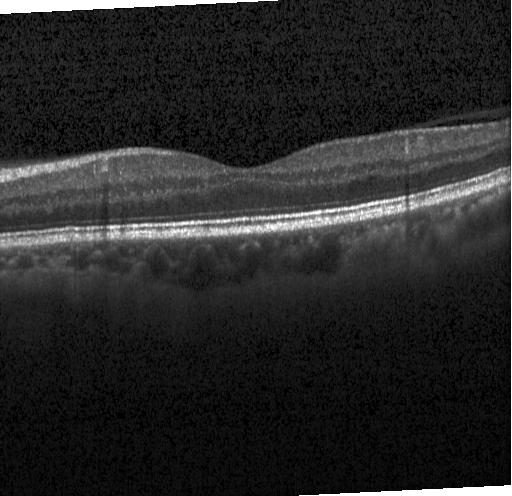
Optical coherence tomography scan · spectral-domain optical coherence tomography · acquired on a Heidelberg Spectralis. Neither CNV, DME, nor drusen.